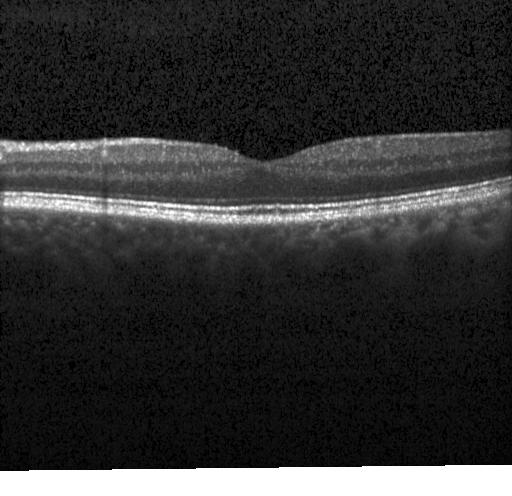
SD-OCT · OCT line scan. Diagnosis: no choroidal neovascularization, diabetic macular edema, or drusen.